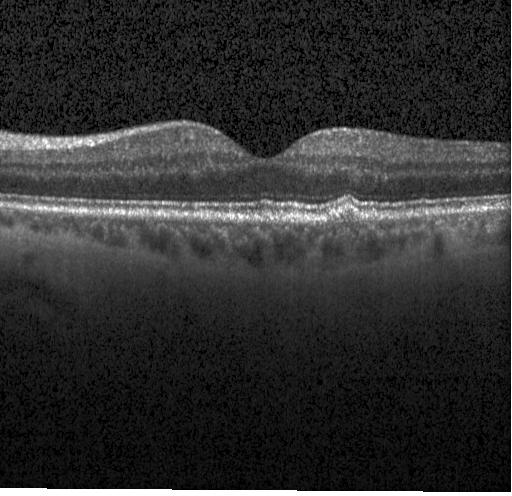

OCT scan showing multiple drusen.